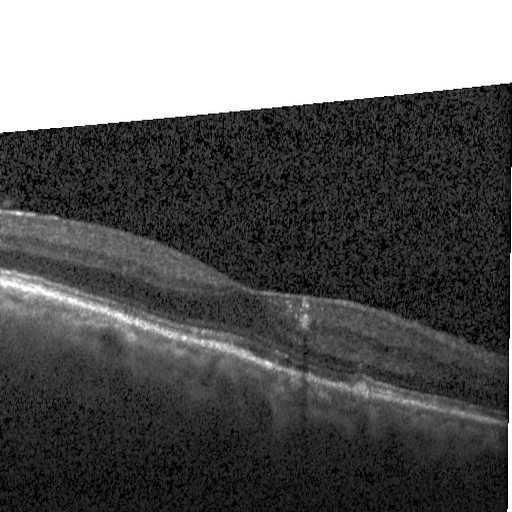 Diagnosis: diabetic macular edema (DME).